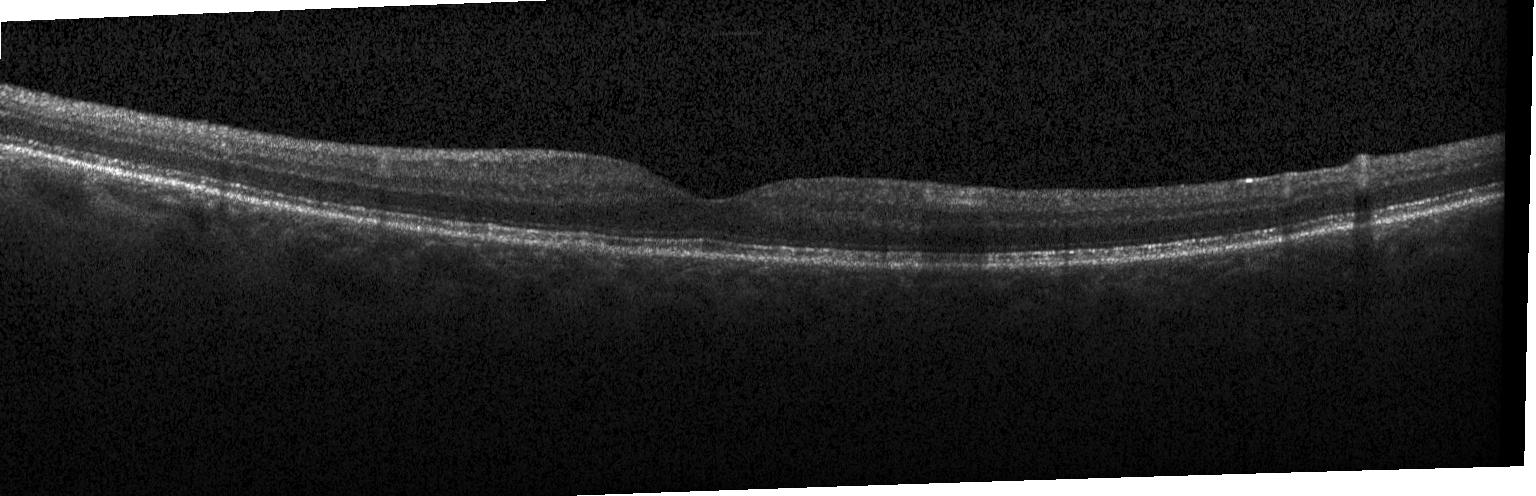

Macular scan. Heidelberg Spectralis OCT system. Retinal OCT B-scan. SD-OCT
This B-scan demonstrates no evidence of choroidal neovascularization, diabetic macular edema, or drusen.